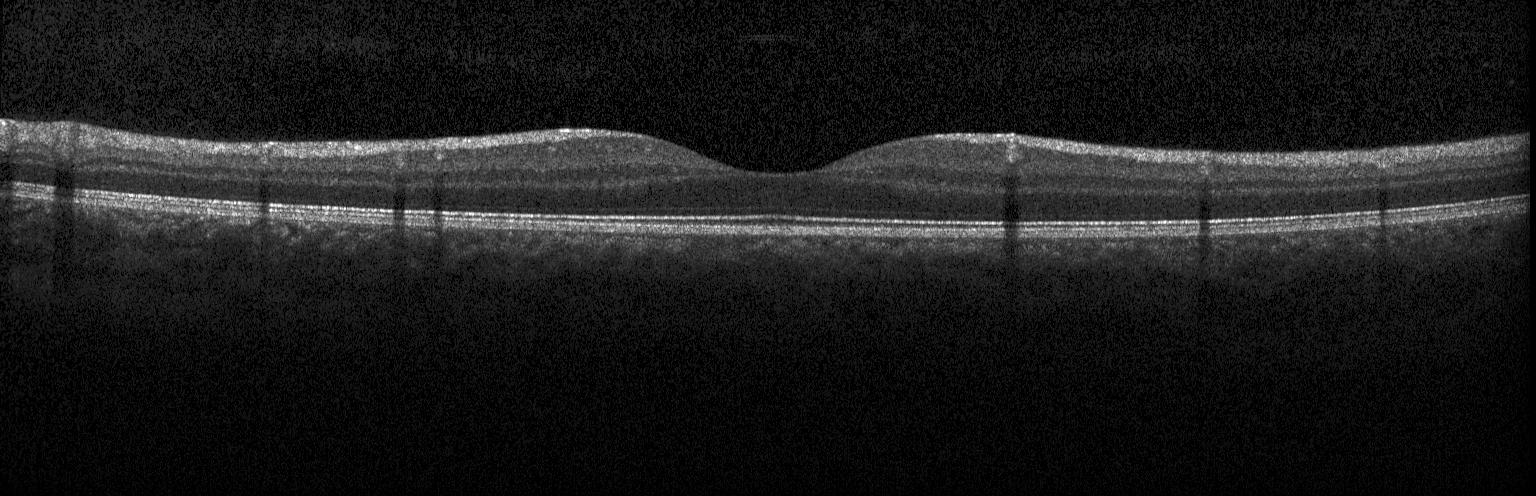 Fovea-centered. Instrument: Heidelberg Spectralis. Retinal OCT B-scan. Spectral-domain OCT
Impression: no evidence of choroidal neovascularization, diabetic macular edema, or drusen.